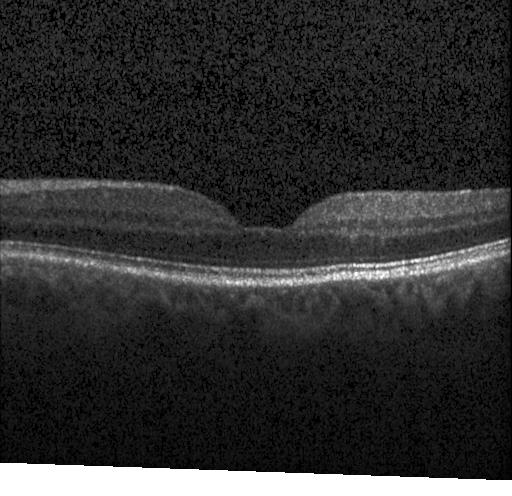

Dx: no evidence of choroidal neovascularization, diabetic macular edema, or drusen.